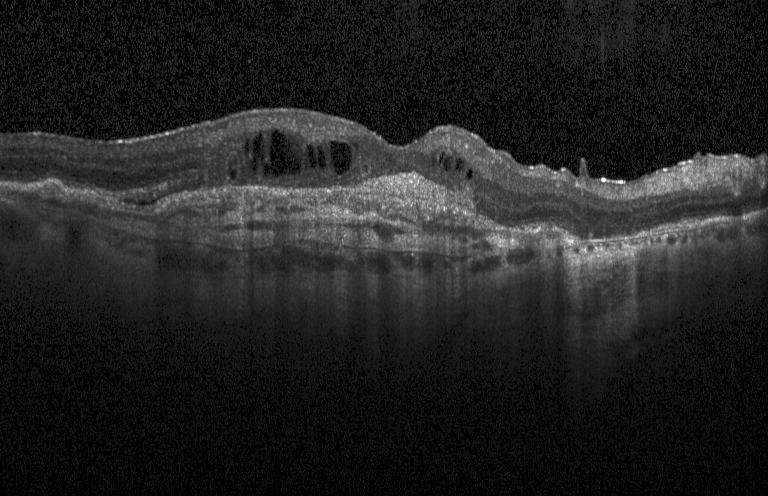
Spectral-domain OCT B-scan: choroidal neovascularization.